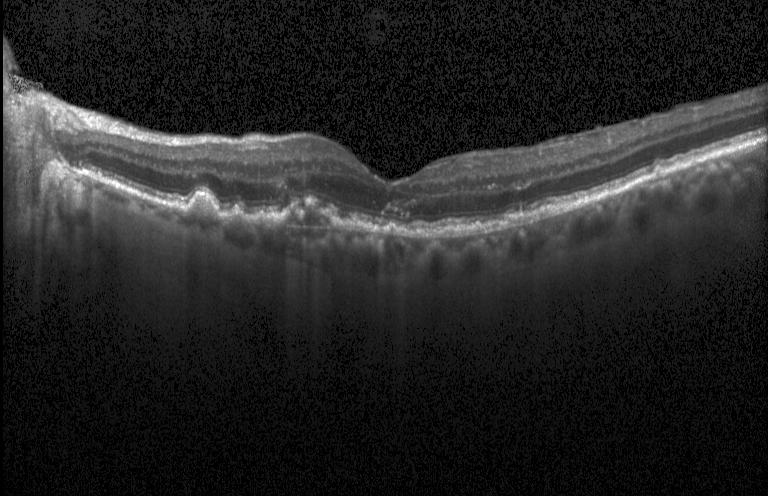

Assessment: choroidal neovascularization.